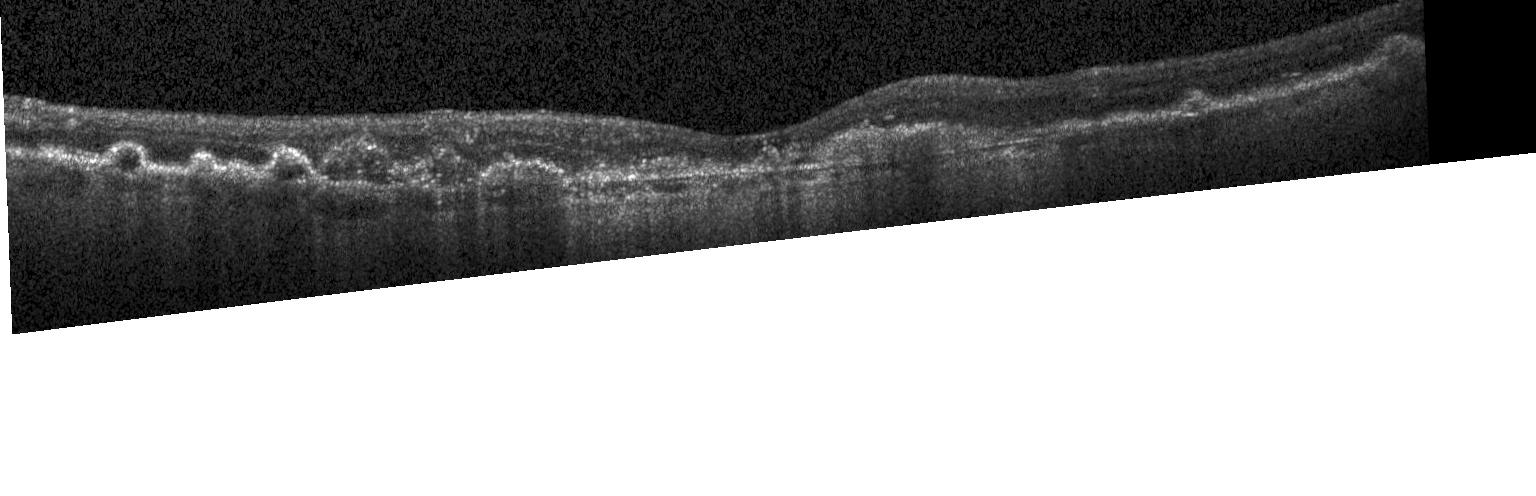
Retinal OCT B-scan · spectral-domain OCT · fovea-centered — Finding: a choroidal neovascular membrane.